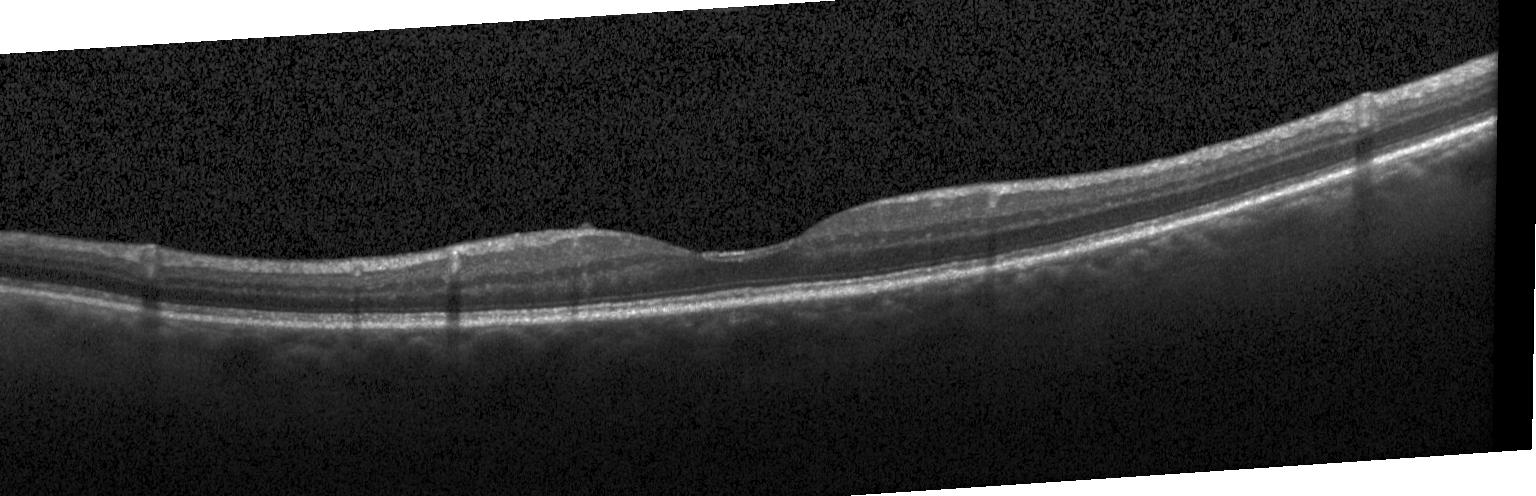
OCT line scan — Assessment: no choroidal neovascularization, no diabetic macular edema, and no drusen.